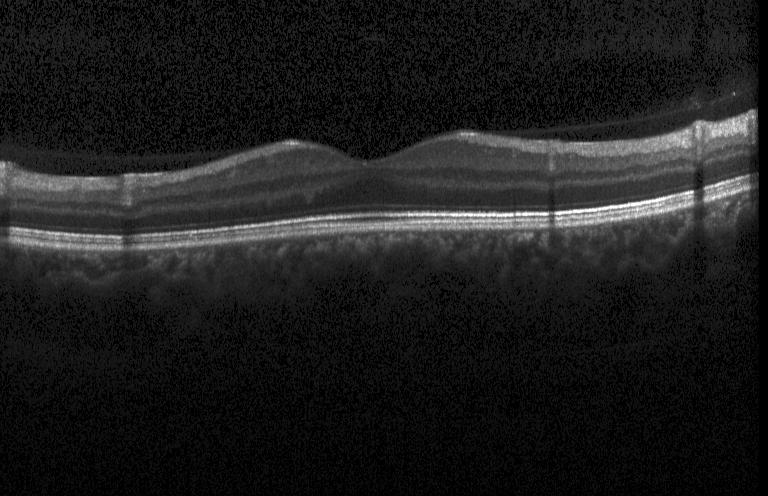 Diagnosis: no choroidal neovascularization, diabetic macular edema, or drusen.